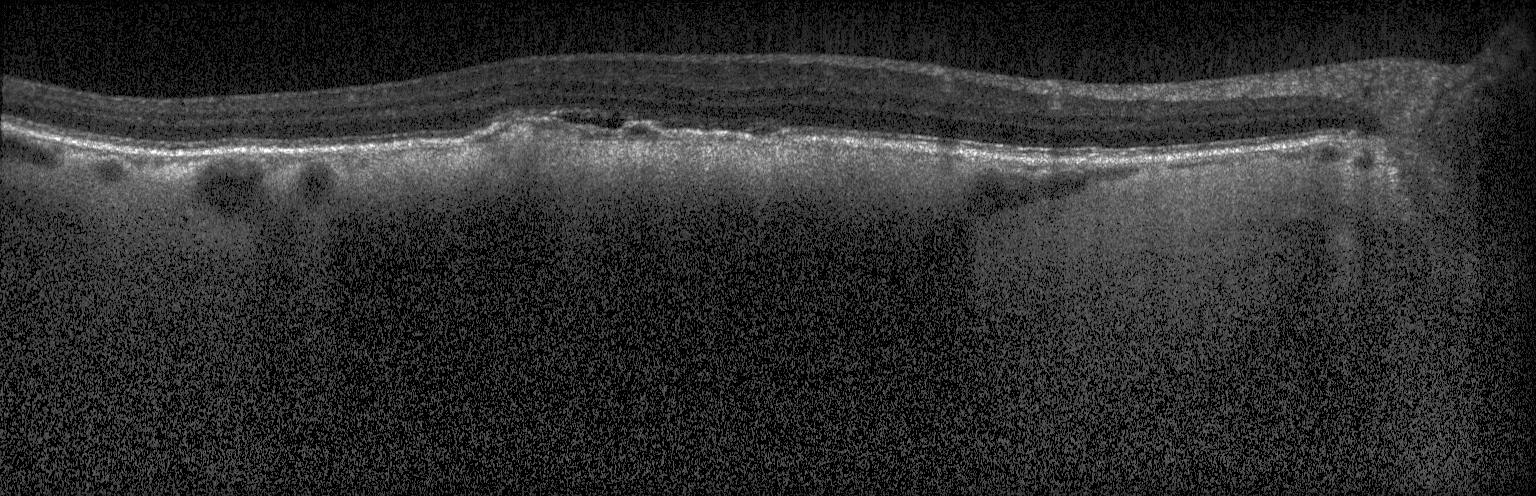

Diagnosis: a choroidal neovascular membrane.